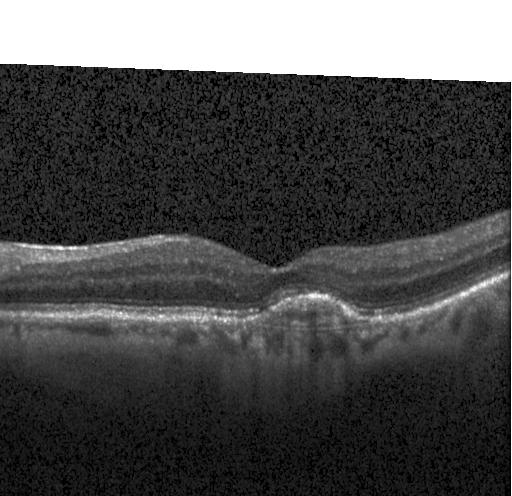

OCT scan showing CNV.